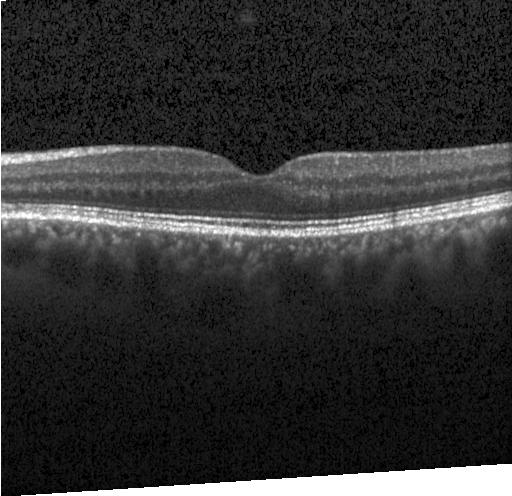

Dx: no evidence of choroidal neovascularization, diabetic macular edema, or drusen.